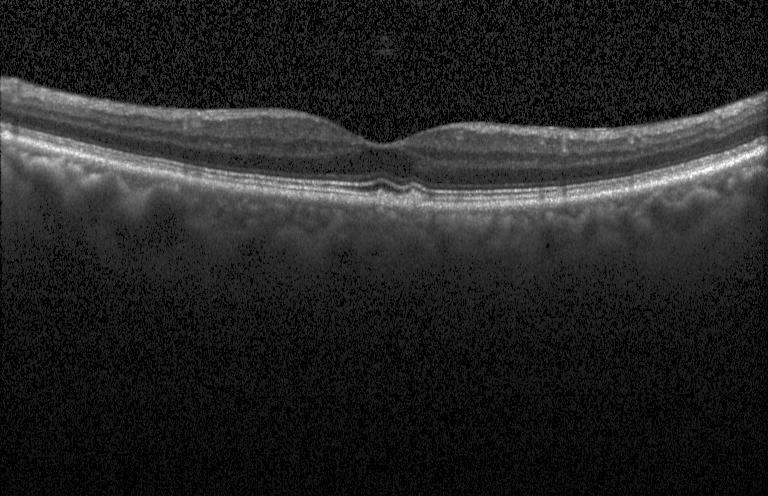

Retinal OCT B-scan. Spectral-domain optical coherence tomography — The scan shows sub-RPE drusenoid deposits.